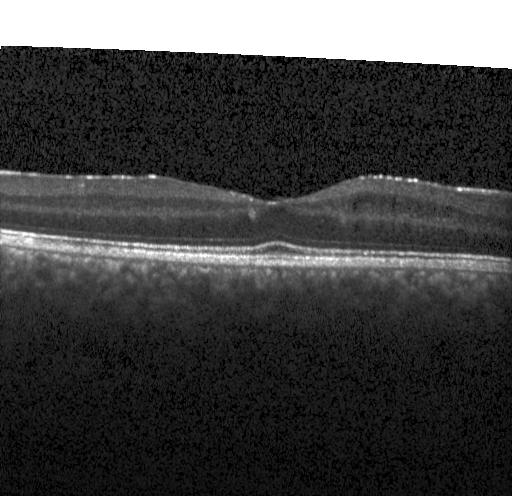

Heidelberg Spectralis; optical coherence tomography B-scan; spectral-domain OCT
Diabetic macular edema.